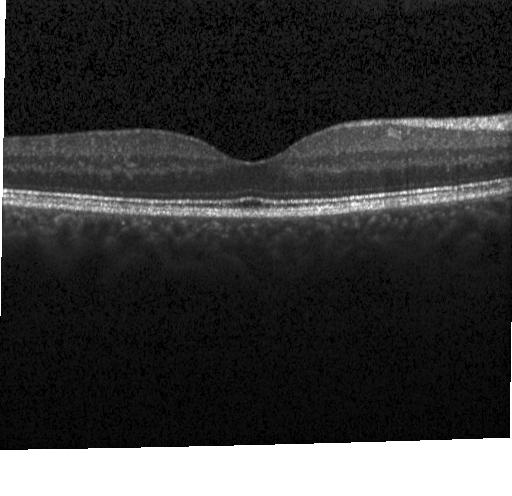

Optical coherence tomography scan — Finding: neither CNV, DME, nor drusen.